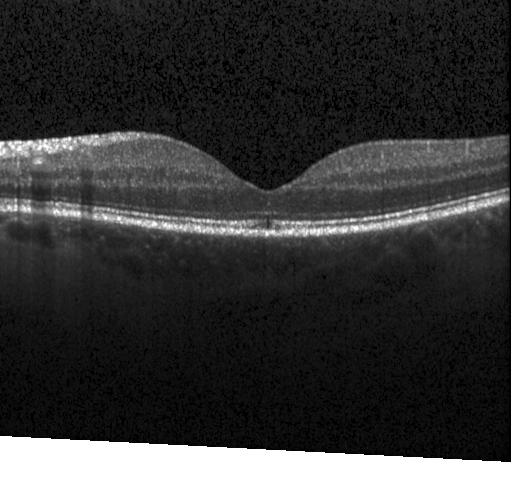
Spectral-domain OCT B-scan: no evidence of CNV, DME, or drusen.